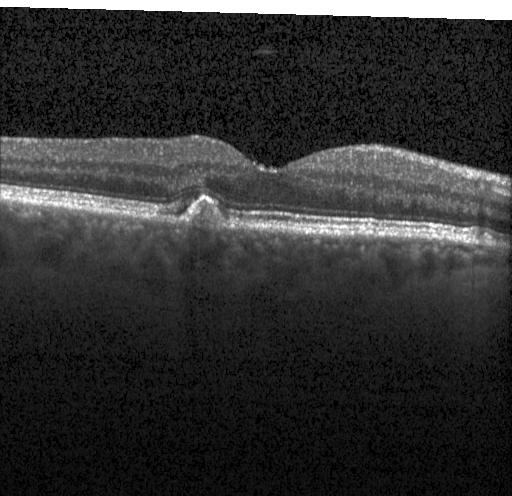
OCT B-scan — Macular OCT: CNV.